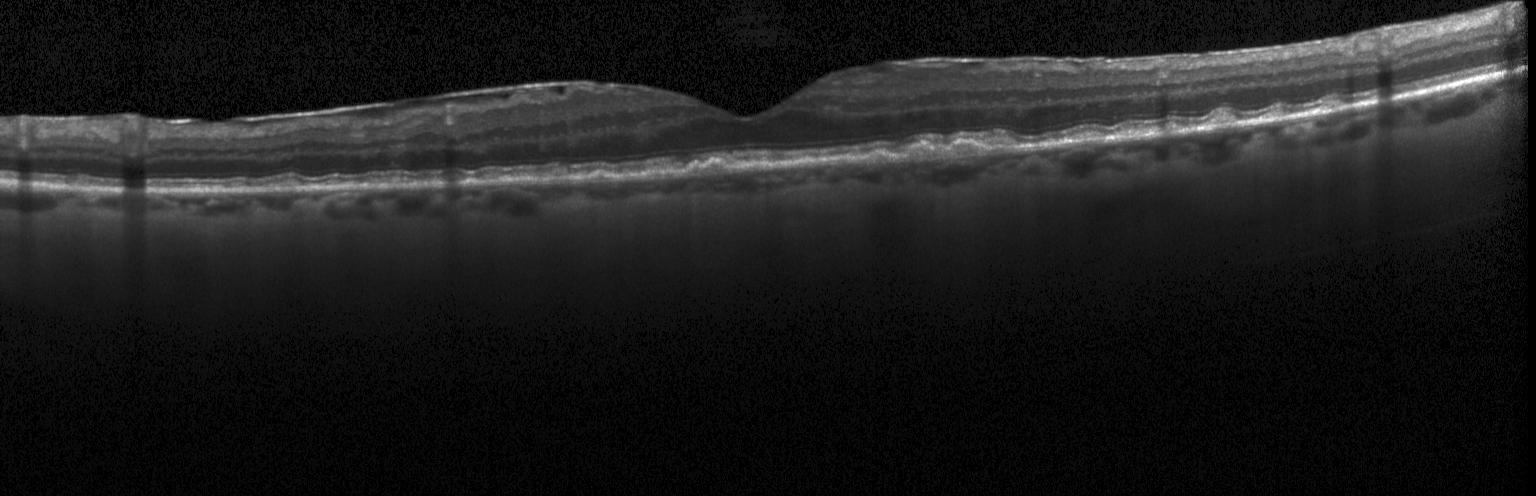

Spectral-domain optical coherence tomography · Heidelberg Spectralis OCT system · horizontal scan through the fovea · OCT B-scan — Assessment: drusen.